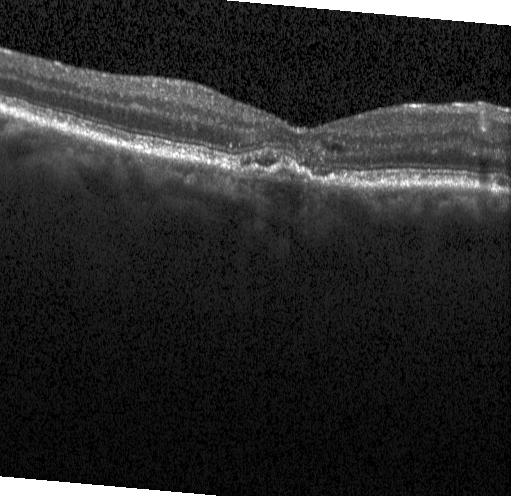

Retinal OCT B-scan — The scan shows choroidal neovascularization (CNV).